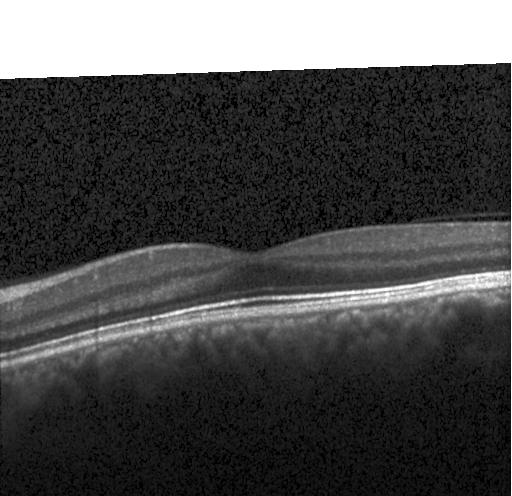
OCT line scan. Spectral-domain optical coherence tomography. Heidelberg Spectralis OCT system. Horizontal scan through the fovea.
Diagnosis: neither CNV, DME, nor drusen.